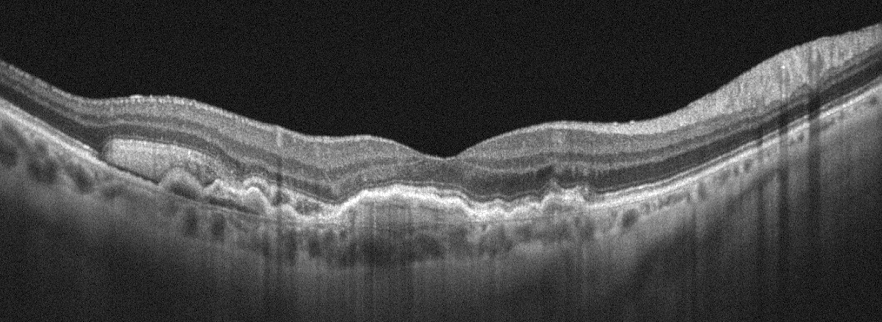

Macular scan; acquired on an Optovue Avanti RTVue XR; optical coherence tomography B-scan
Diagnosis: AMD.